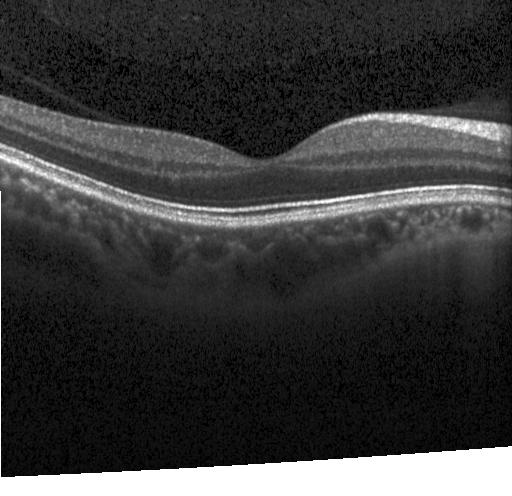
No evidence of choroidal neovascularization, diabetic macular edema, or drusen.